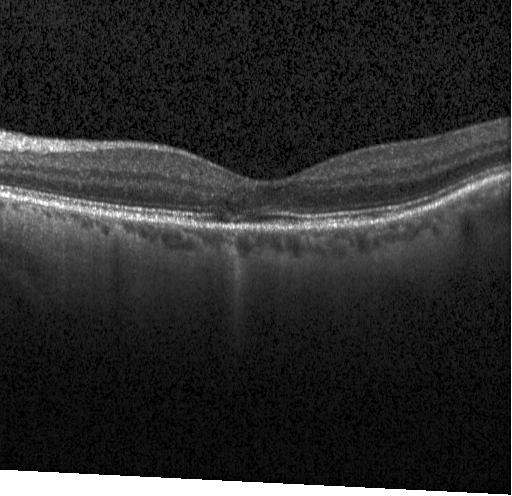
SD-OCT. Retinal OCT cross-section. Heidelberg Spectralis. Through the macula. Finding: neither choroidal neovascularization, diabetic macular edema, nor drusen.